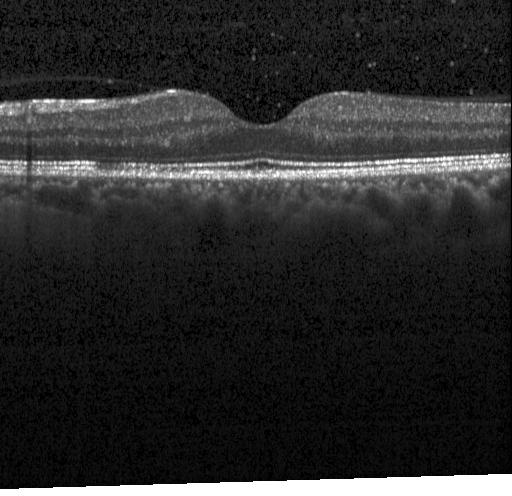

Retinal OCT B-scan — This B-scan demonstrates no choroidal neovascularization, no diabetic macular edema, and no drusen.